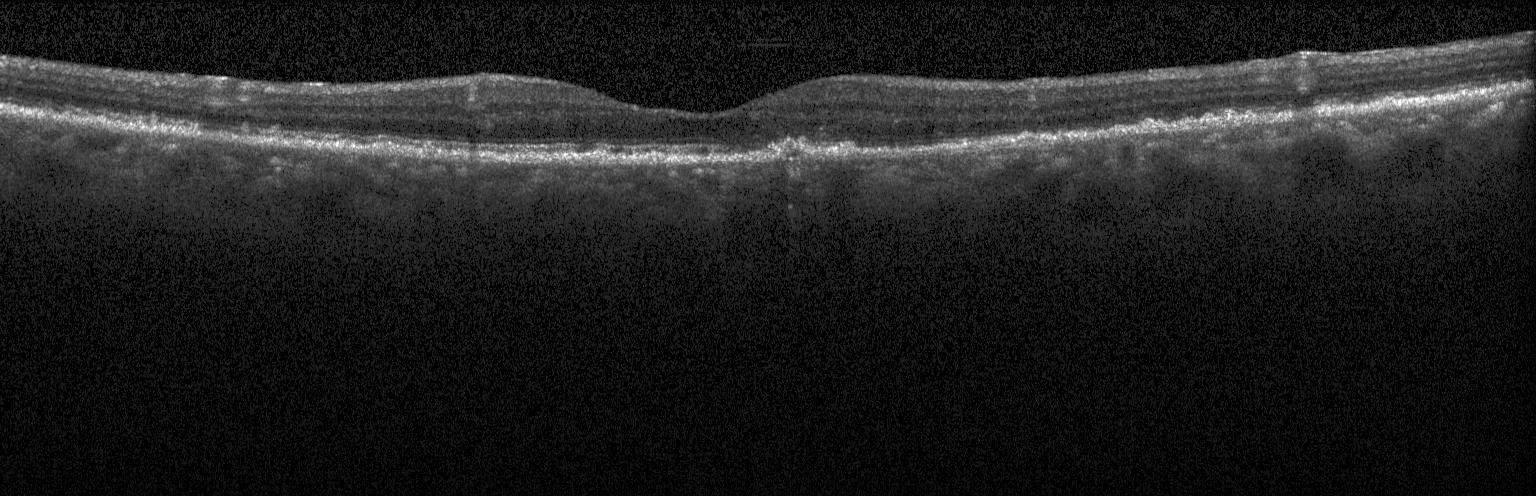

Retinal OCT cross-section. Centered on the fovea. Heidelberg Spectralis.
Assessment: sub-RPE drusenoid deposits.